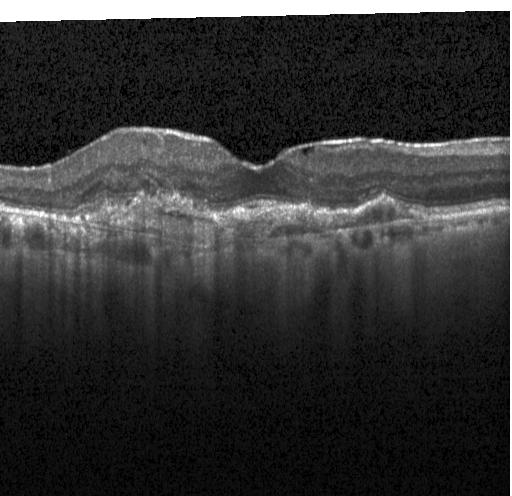 Optical coherence tomography scan.
Diagnosis: a choroidal neovascular membrane.